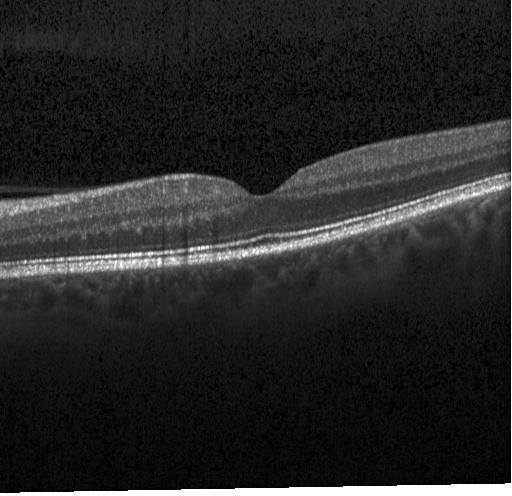
OCT line scan.
Assessment: no CNV, DME, or drusen.